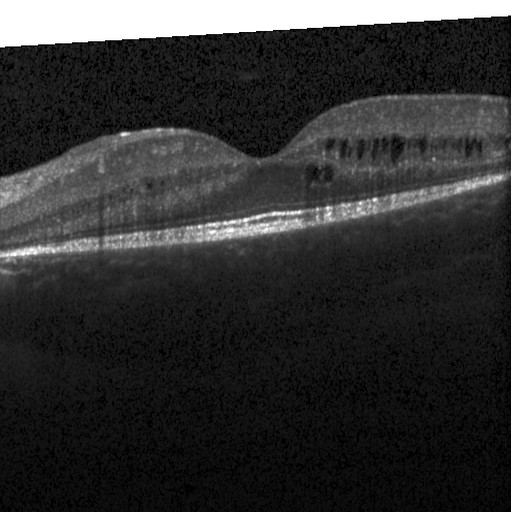 Impression: diabetic macular edema.